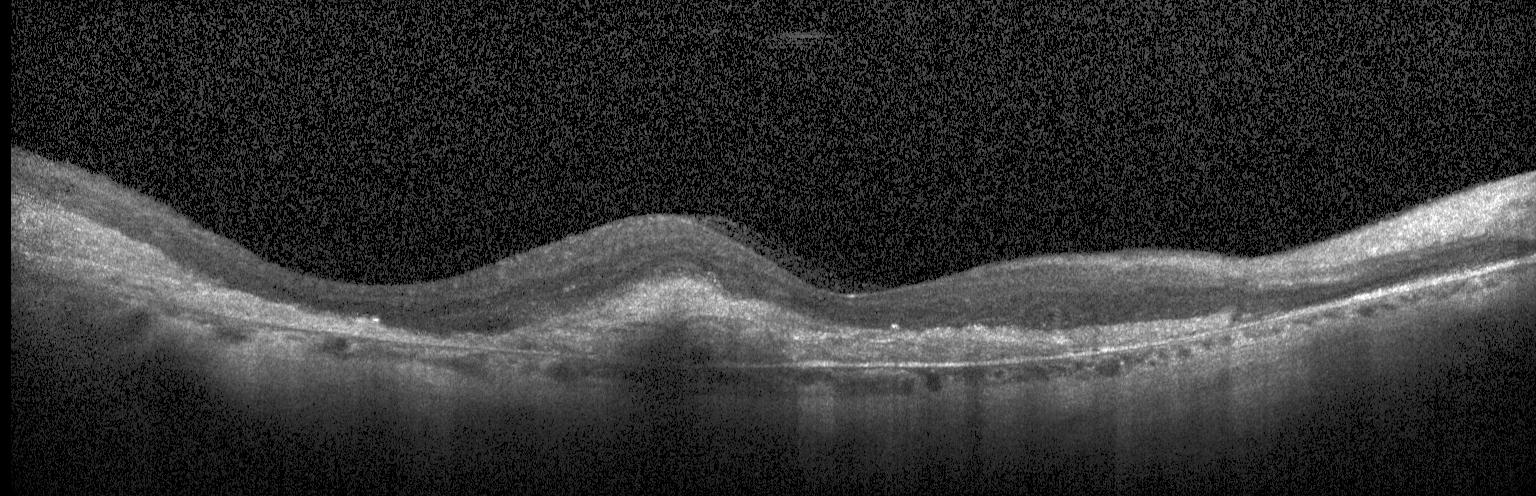
Assessment: a choroidal neovascular membrane.